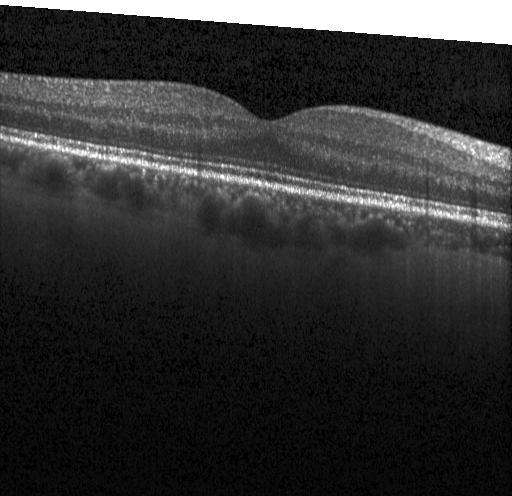 OCT B-scan. Horizontal scan through the fovea. Heidelberg Spectralis OCT system — The scan shows neither choroidal neovascularization, diabetic macular edema, nor drusen.